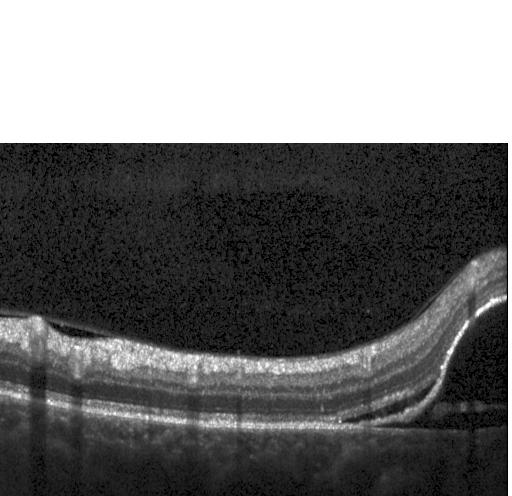
Instrument: Heidelberg Spectralis. Spectral-domain OCT. OCT line scan.
Diagnosis: choroidal neovascularization.